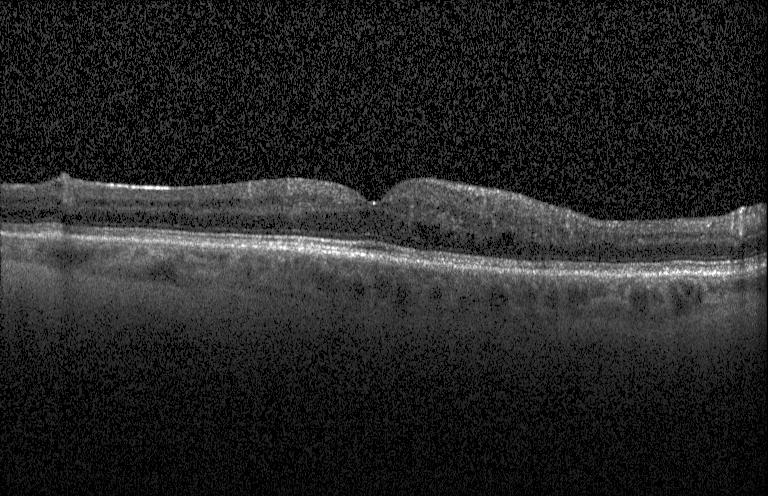 Diagnosis: DME.